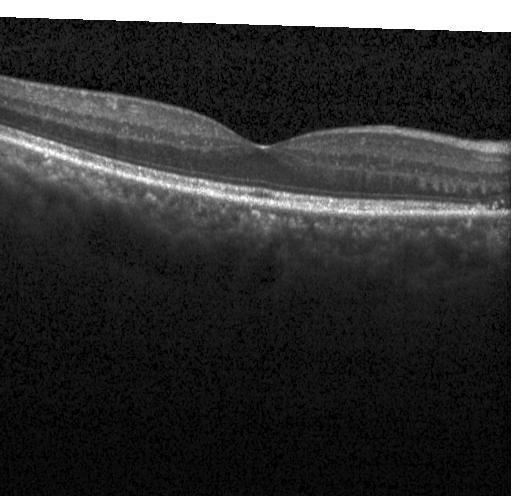

Dx: no CNV, no DME, and no drusen.